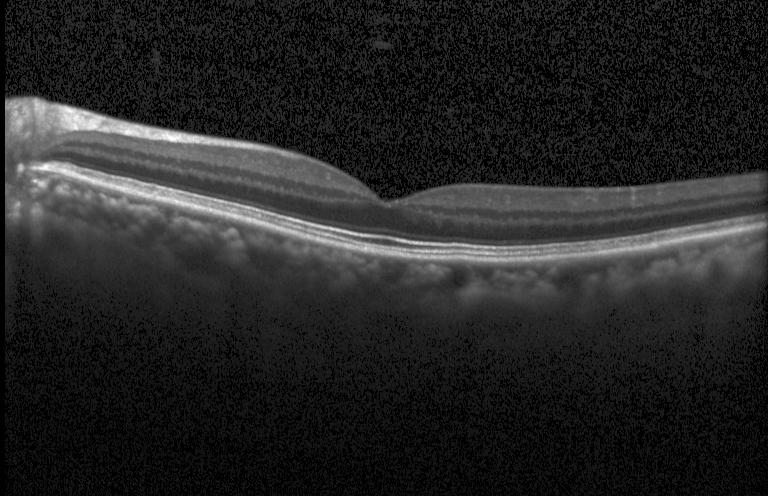 OCT B-scan — No CNV, DME, or drusen.